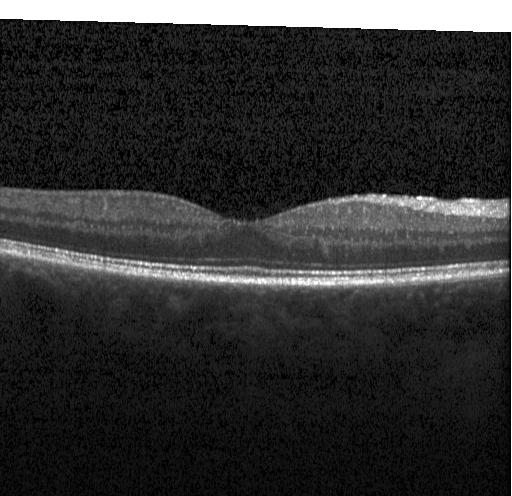

Centered on the fovea. Spectral-domain OCT. Instrument: Heidelberg Spectralis. OCT line scan. No evidence of CNV, DME, or drusen.